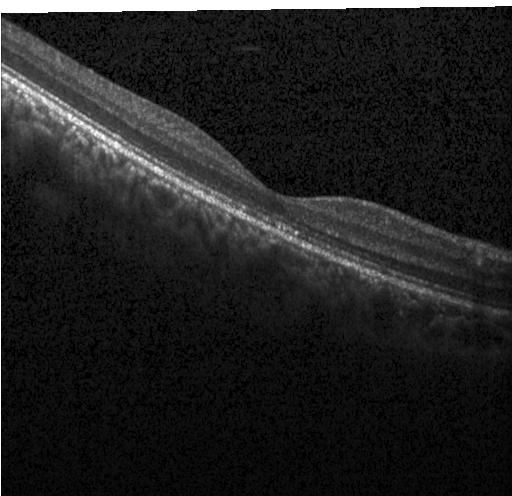

No choroidal neovascularization, diabetic macular edema, or drusen.